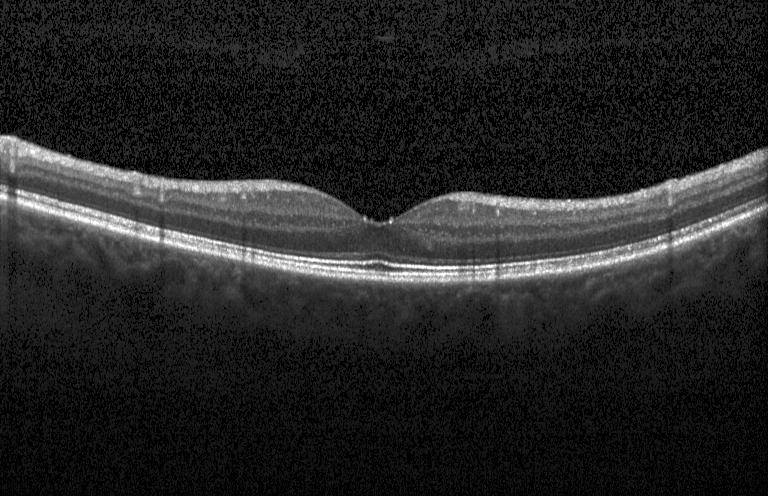

Optical coherence tomography scan.
No choroidal neovascularization, diabetic macular edema, or drusen.